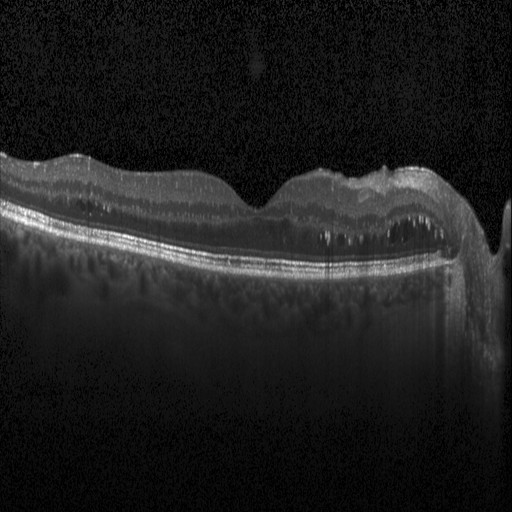
Fovea-centered. OCT line scan. SD-OCT. Finding: DME.